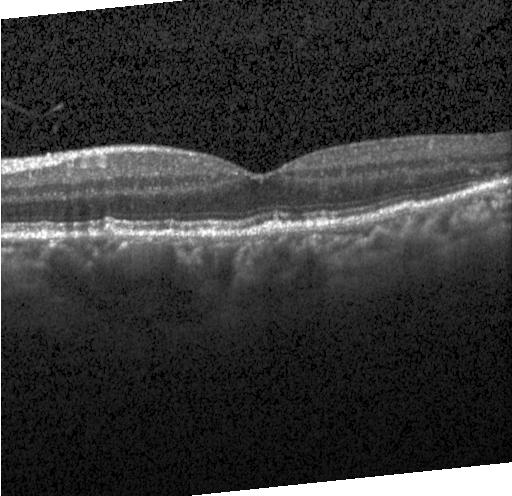

Centered on the fovea, instrument: Heidelberg Spectralis, retinal OCT cross-section
The scan shows multiple drusen.